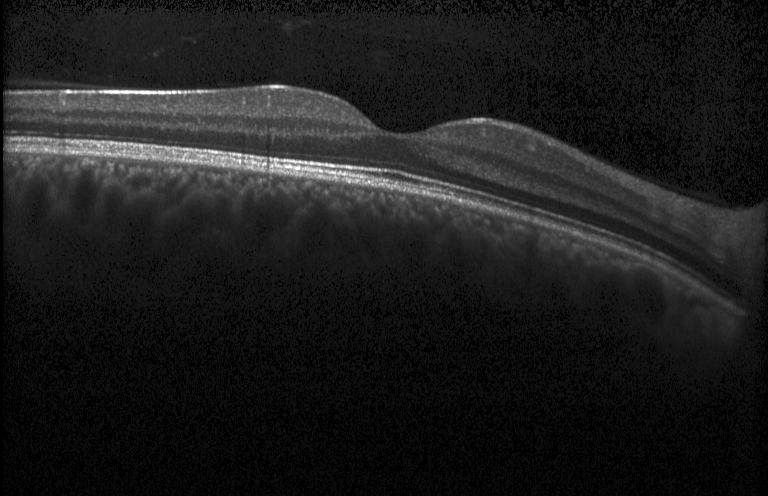 OCT B-scan. Diagnosis: no evidence of choroidal neovascularization, diabetic macular edema, or drusen.